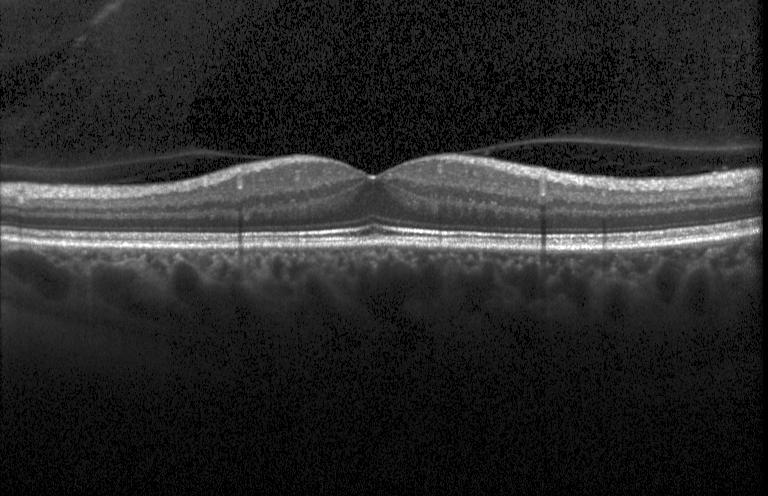
Centered on the fovea · retinal OCT B-scan — Diagnosis: neither choroidal neovascularization, diabetic macular edema, nor drusen.